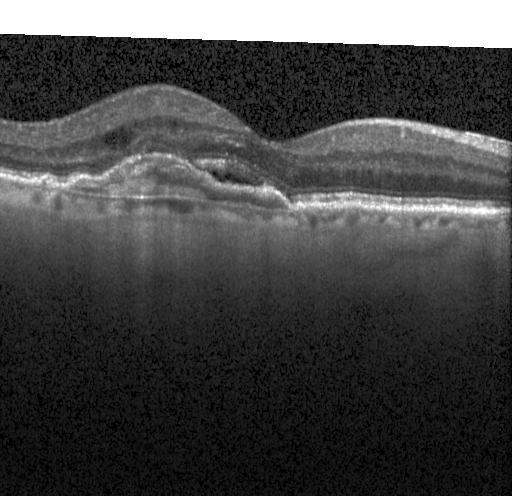 OCT finding: CNV.